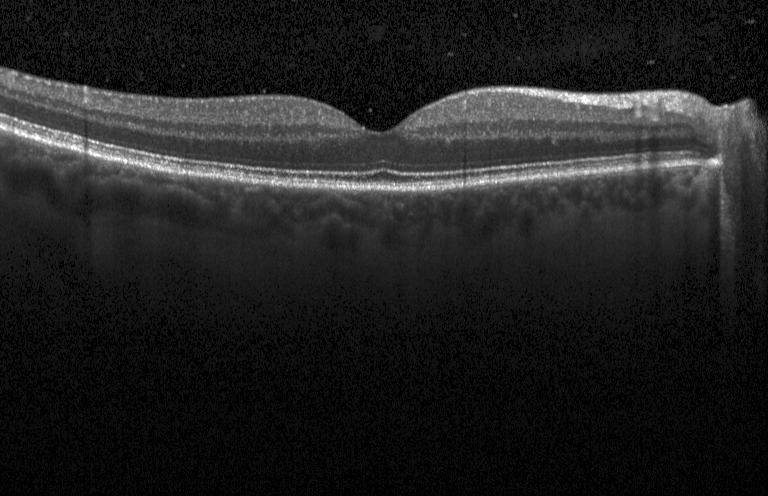 Heidelberg Spectralis; OCT line scan; fovea-centered. Diagnosis: no CNV, no DME, and no drusen.